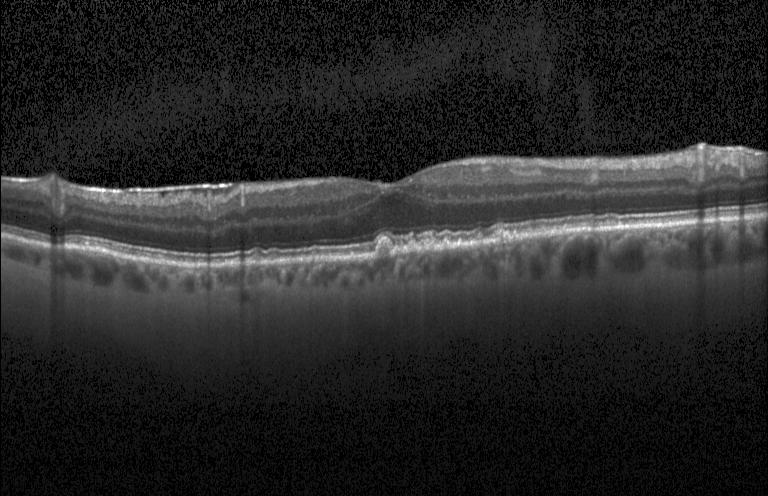

OCT B-scan, Heidelberg Spectralis.
Finding: sub-RPE drusenoid deposits.